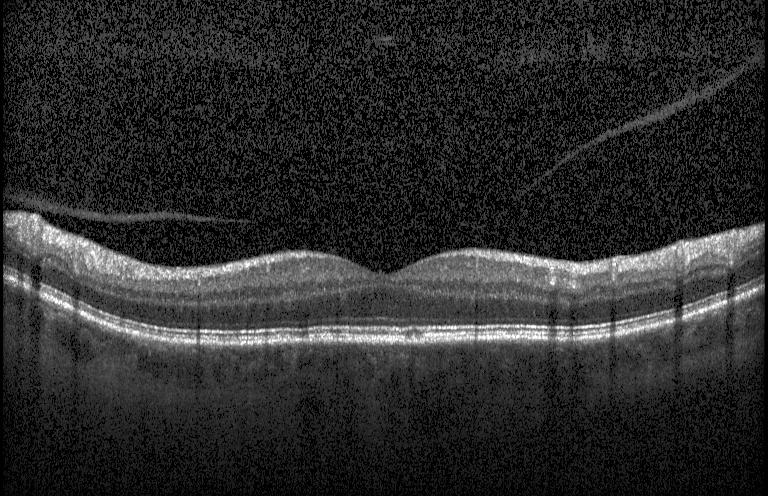
SD-OCT · centered on the fovea · OCT B-scan. OCT finding: no choroidal neovascularization, no diabetic macular edema, and no drusen.